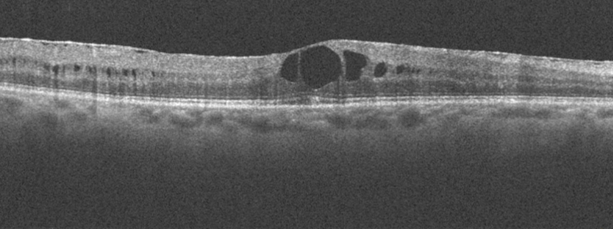

OCT line scan — This B-scan demonstrates DME.